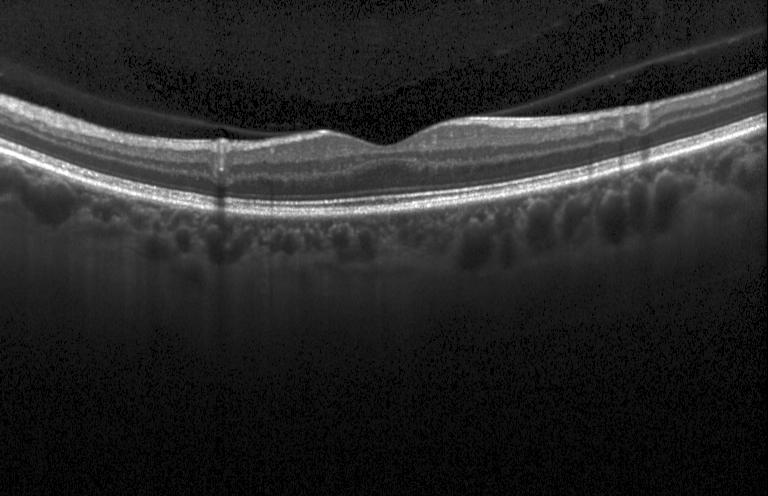 Instrument: Heidelberg Spectralis; SD-OCT; optical coherence tomography B-scan. Assessment: no evidence of CNV, DME, or drusen.